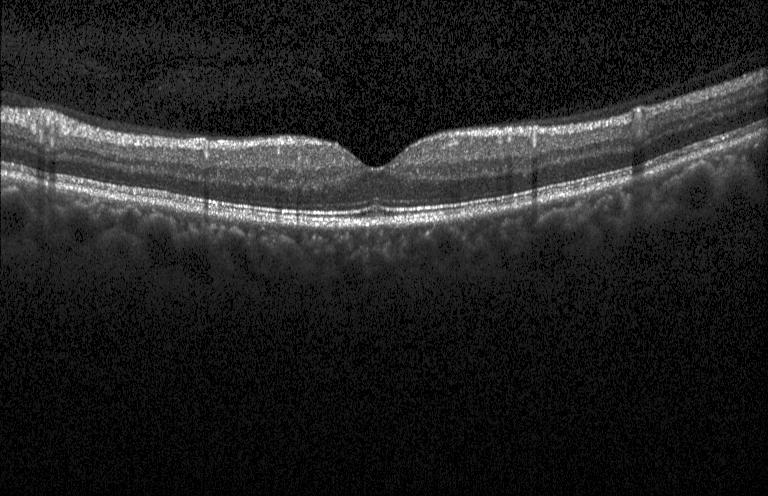

OCT line scan.
Finding: no evidence of choroidal neovascularization, diabetic macular edema, or drusen.